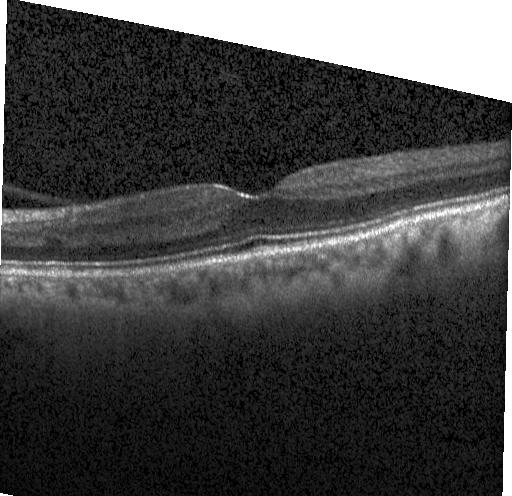
Optical coherence tomography B-scan
No choroidal neovascularization, diabetic macular edema, or drusen.